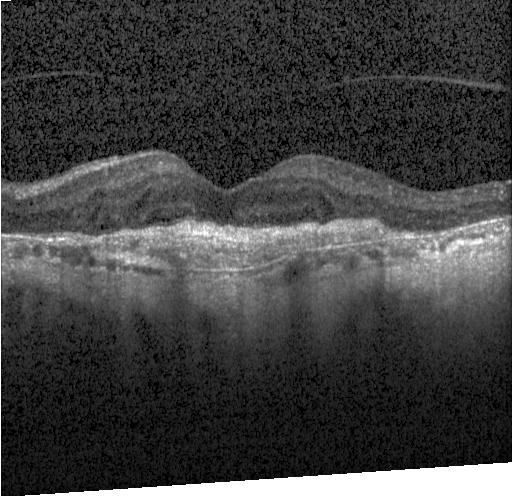
Optical coherence tomography scan
Impression: a choroidal neovascular membrane.